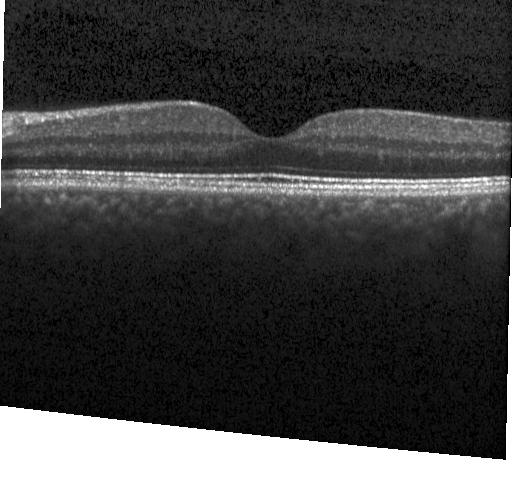

Retinal OCT B-scan; fovea-centered; spectral-domain optical coherence tomography
Finding: neither choroidal neovascularization, diabetic macular edema, nor drusen.